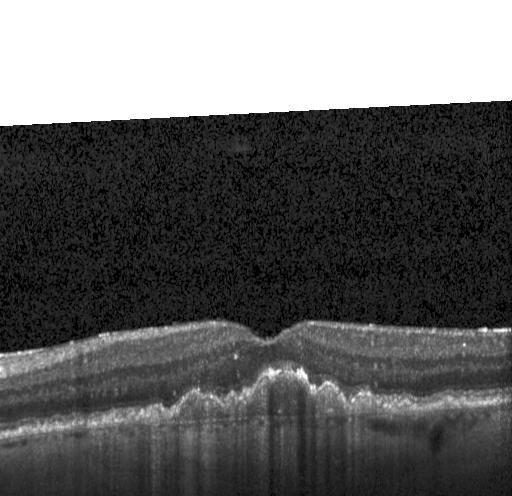 SD-OCT, retinal OCT cross-section, horizontal scan through the fovea.
Diagnosis: a choroidal neovascular membrane.